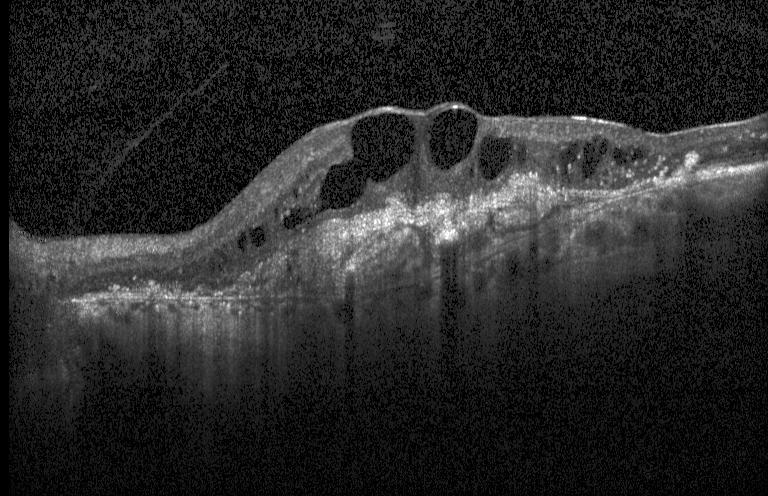
Retinal OCT cross-section showing choroidal neovascularization (CNV).